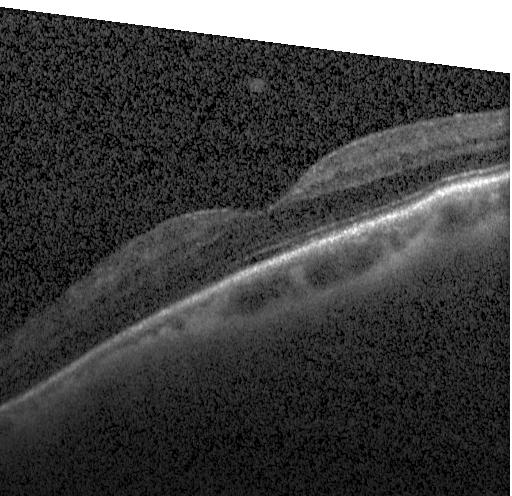
Retinal OCT cross-section.
Impression: no choroidal neovascularization, diabetic macular edema, or drusen.